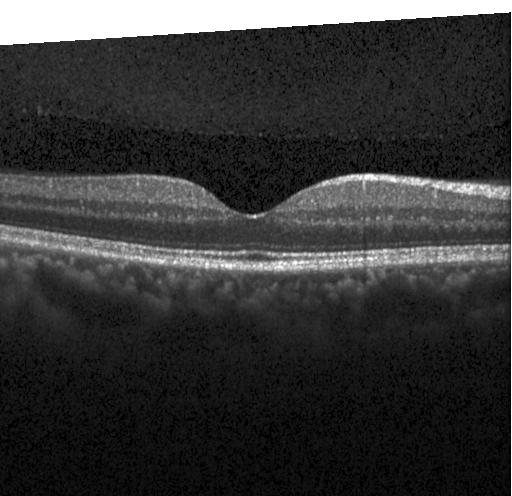

OCT B-scan. Spectral-domain optical coherence tomography. Acquired on a Heidelberg Spectralis. Macular scan — Assessment: no evidence of CNV, DME, or drusen.